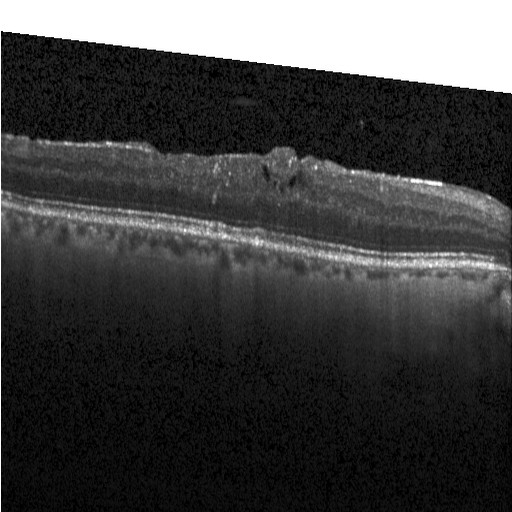
Horizontal scan through the fovea · acquired on a Heidelberg Spectralis · spectral-domain optical coherence tomography · retinal OCT cross-section.
Impression: diabetic macular edema (DME).